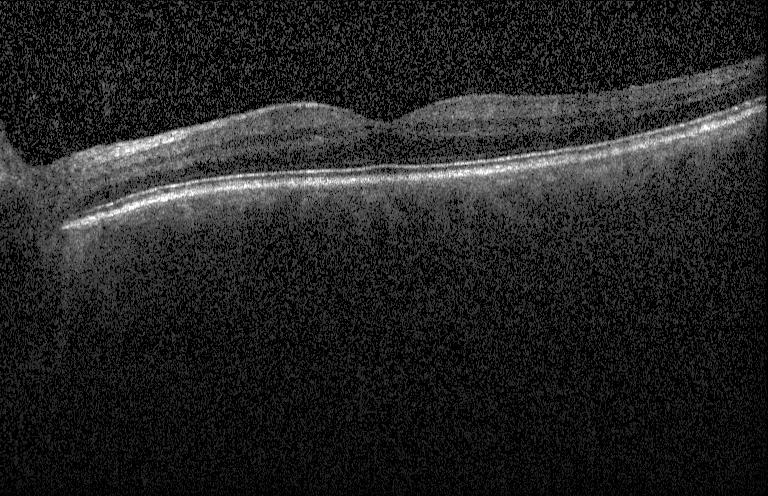

OCT B-scan showing no choroidal neovascularization, no diabetic macular edema, and no drusen.